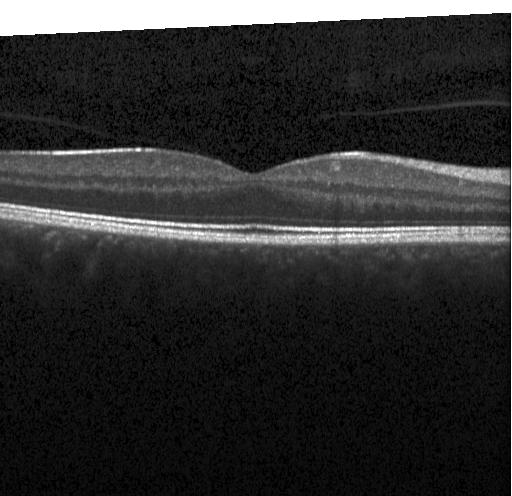 OCT finding: no choroidal neovascularization, diabetic macular edema, or drusen.